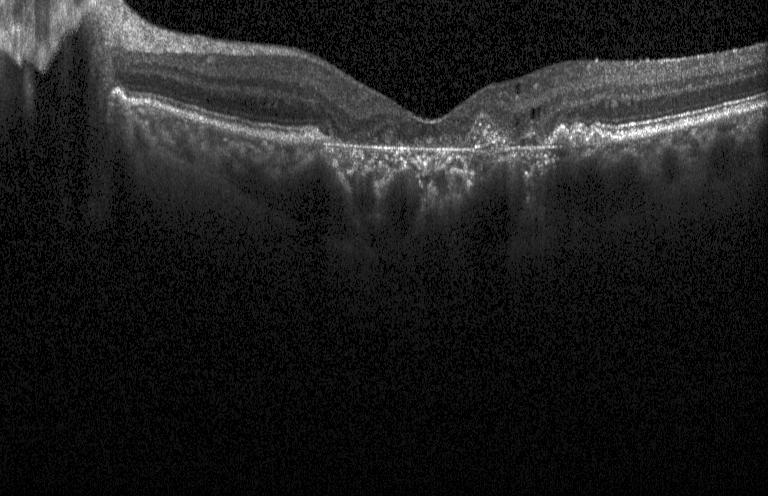

OCT line scan. Centered on the fovea — Finding: a choroidal neovascular membrane.